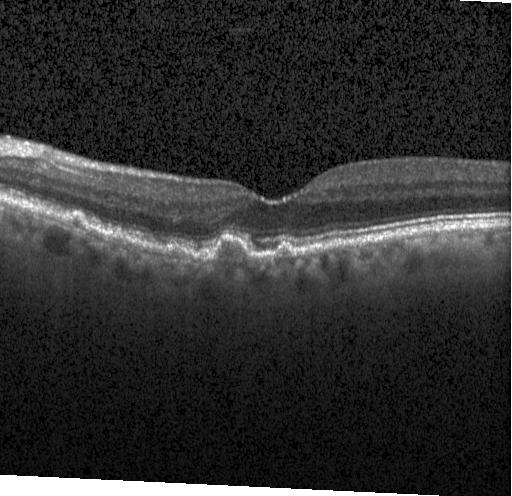
Fovea-centered. Optical coherence tomography B-scan.
This B-scan demonstrates drusen.